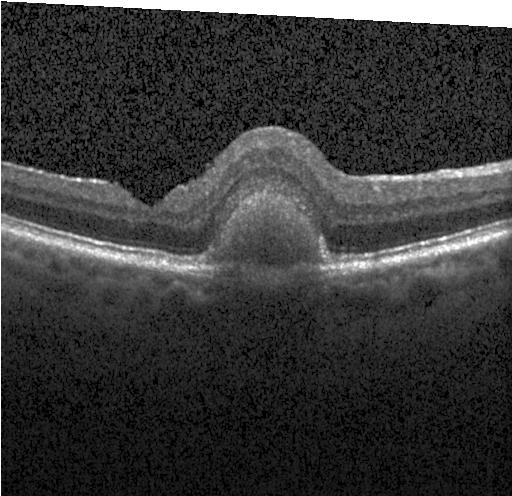

Macular scan, OCT B-scan — Impression: a choroidal neovascular membrane.